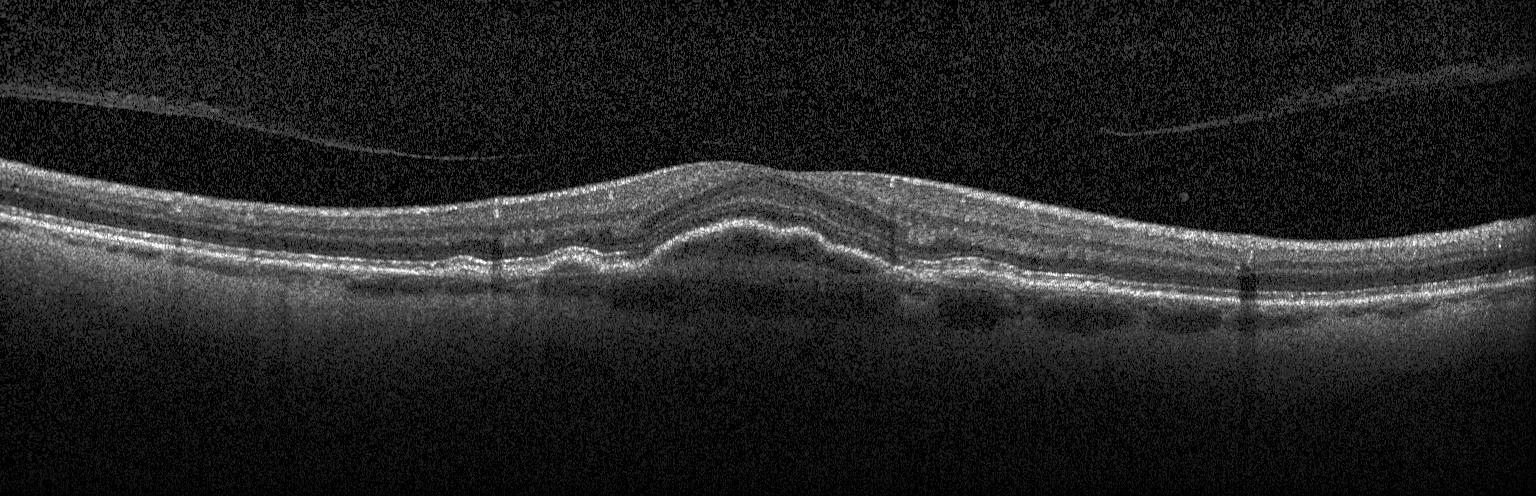
Impression: a choroidal neovascular membrane.